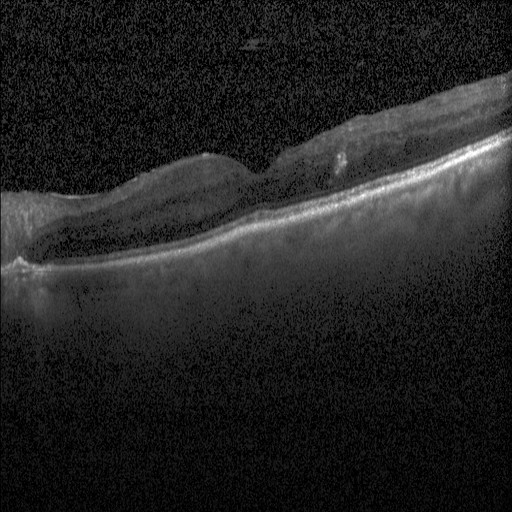
Spectral-domain OCT · horizontal scan through the fovea · optical coherence tomography B-scan · Heidelberg Spectralis — Assessment: diabetic macular edema.